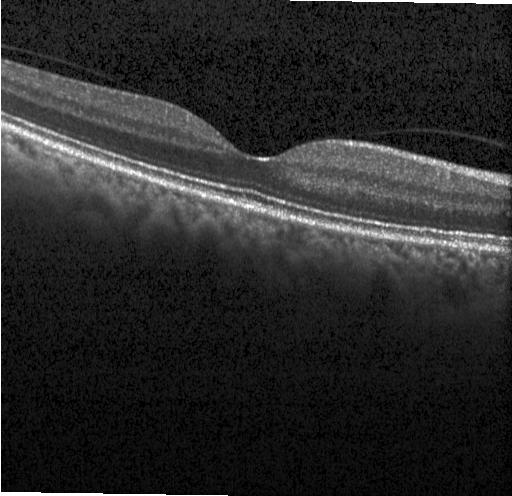 Optical coherence tomography scan, spectral-domain optical coherence tomography.
Finding: no choroidal neovascularization, no diabetic macular edema, and no drusen.